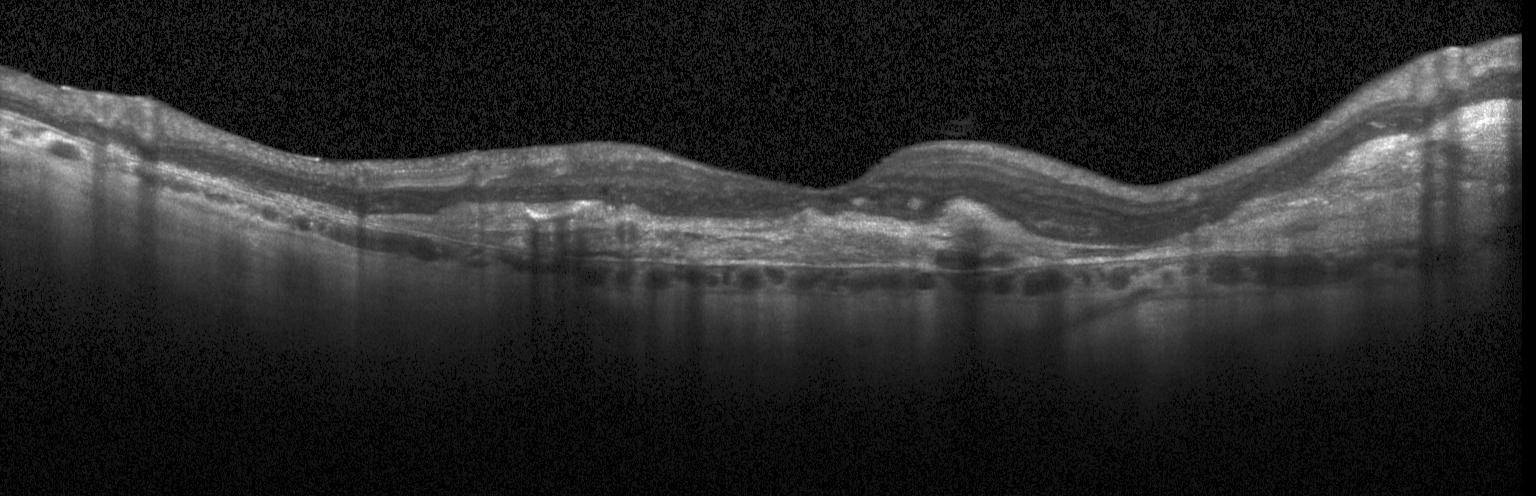 Diagnosis: choroidal neovascularization.